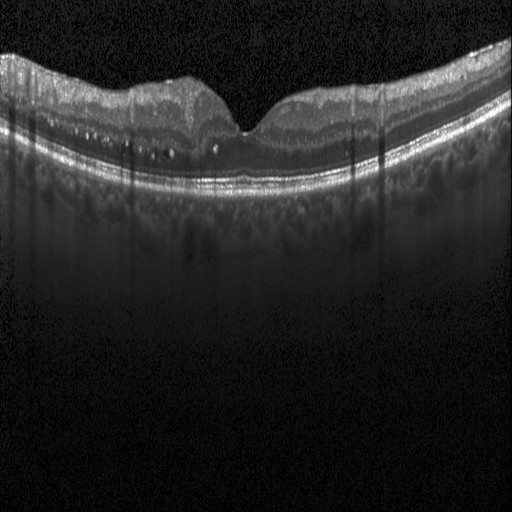

Dx: diabetic macular edema (DME).